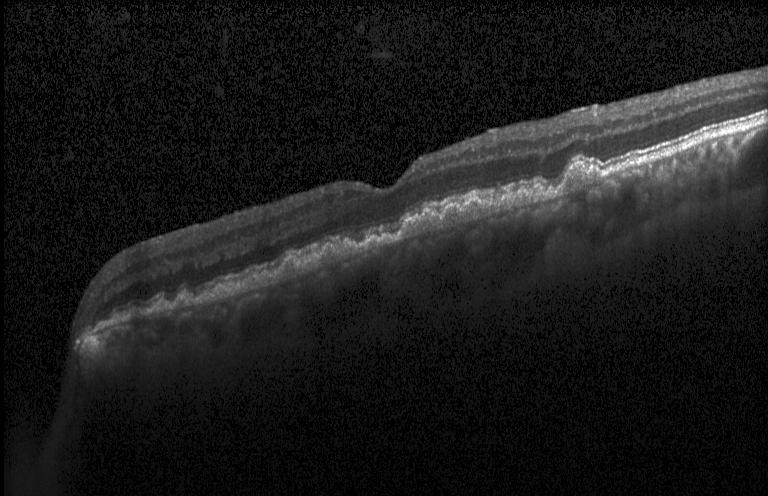 Diagnosis: a choroidal neovascular membrane.